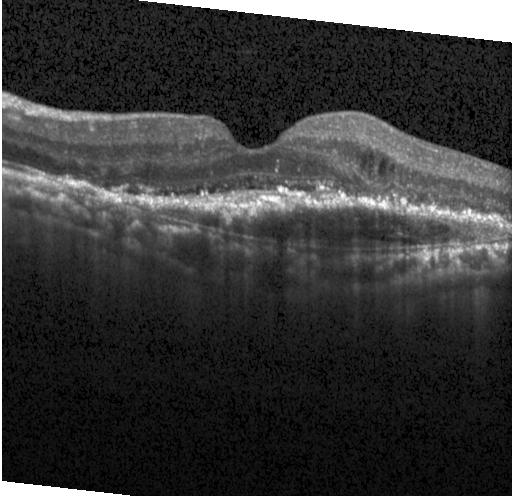
Horizontal scan through the fovea · acquired on a Heidelberg Spectralis · OCT line scan · spectral-domain OCT.
This B-scan demonstrates a choroidal neovascular membrane.